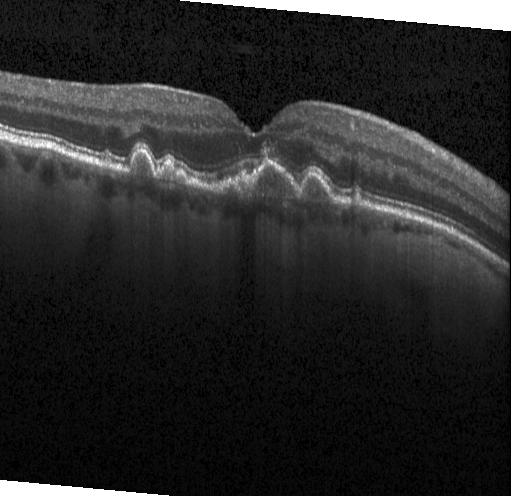

SD-OCT. Retinal OCT cross-section. Heidelberg Spectralis. OCT finding: drusen.